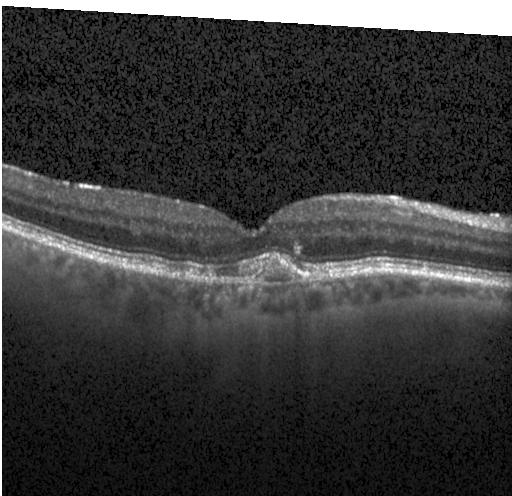
Spectral-domain OCT B-scan: a choroidal neovascular membrane.